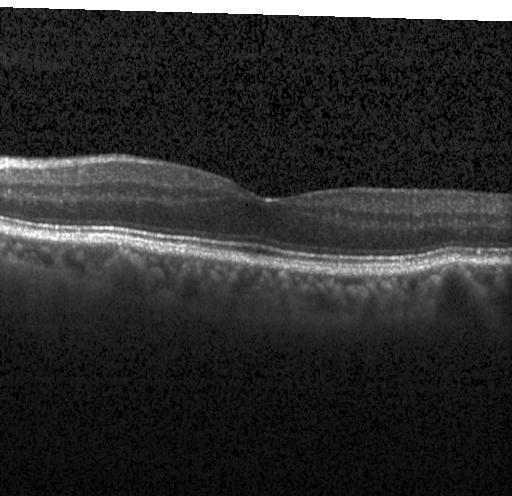 Assessment: no CNV, no DME, and no drusen.